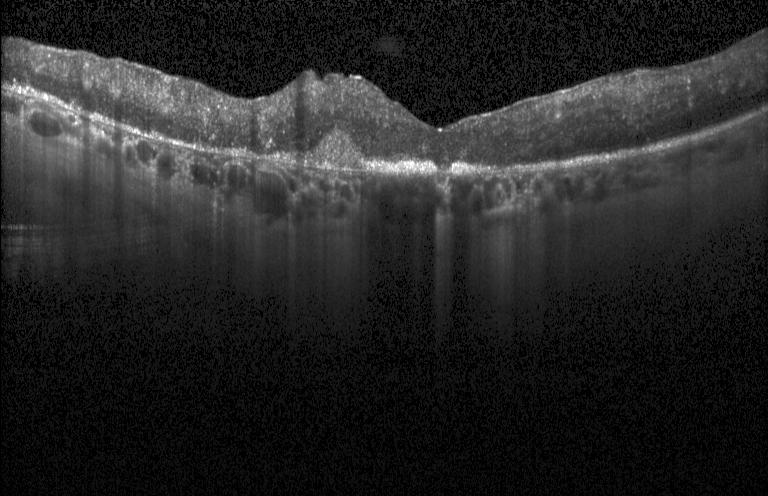 Spectral-domain OCT. Heidelberg Spectralis. Horizontal scan through the fovea. Retinal OCT B-scan. OCT finding: choroidal neovascularization (CNV).